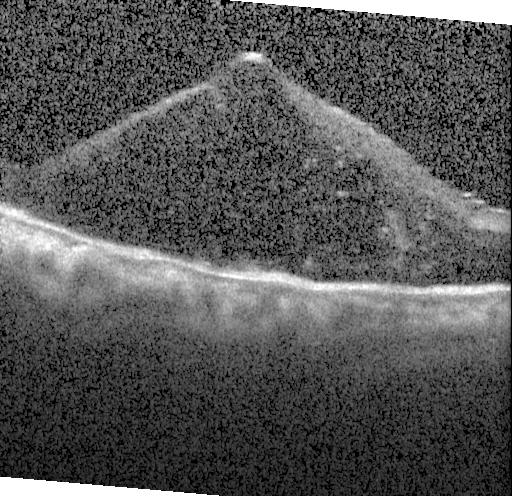 Retinal OCT cross-section; horizontal scan through the fovea; Heidelberg Spectralis OCT system
Diagnosis: diabetic macular edema (DME).